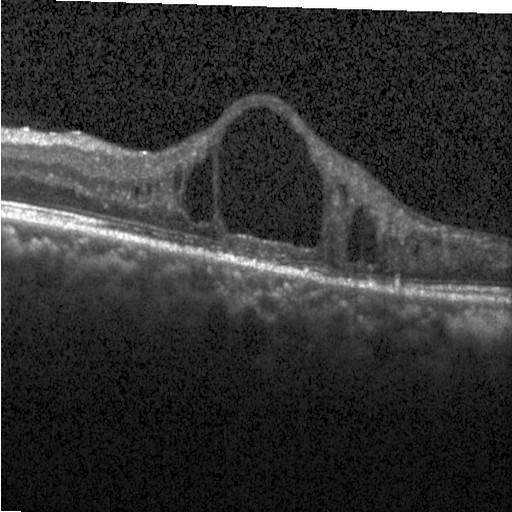 SD-OCT; OCT B-scan. Diagnosis: diabetic macular edema (DME).